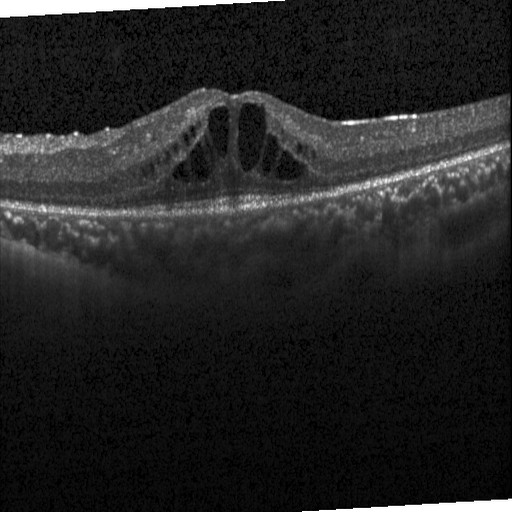
Diagnosis: DME.